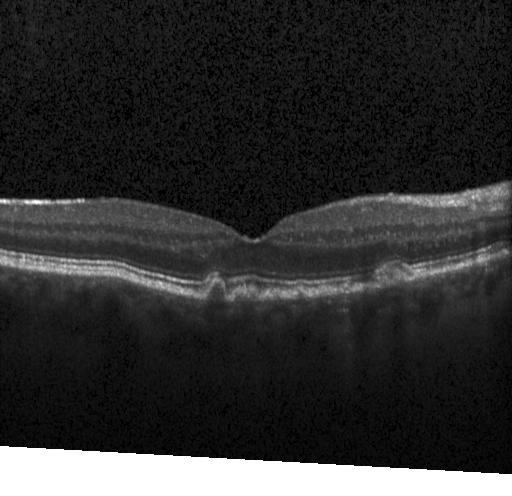

Finding: choroidal neovascularization.